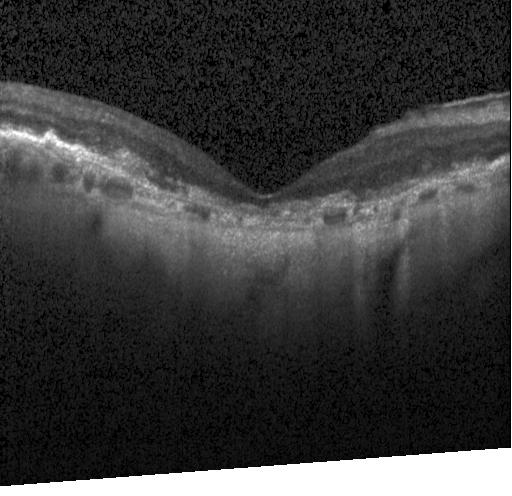 OCT line scan
The scan shows a choroidal neovascular membrane.